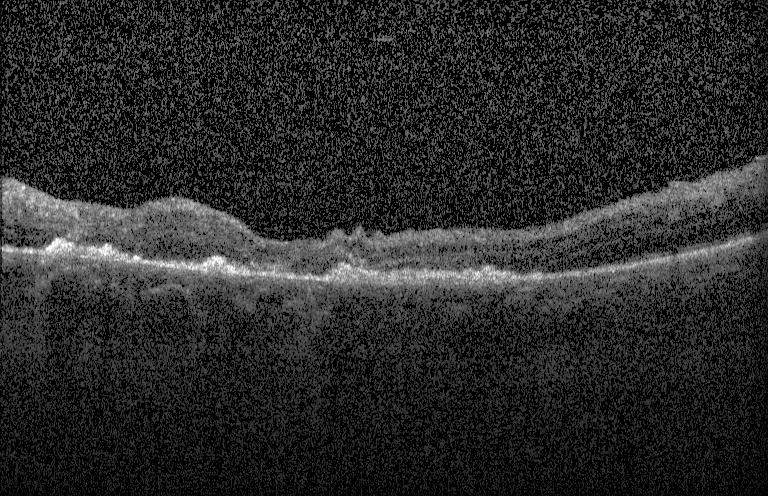
Optical coherence tomography B-scan; acquired on a Heidelberg Spectralis
Finding: choroidal neovascularization (CNV).